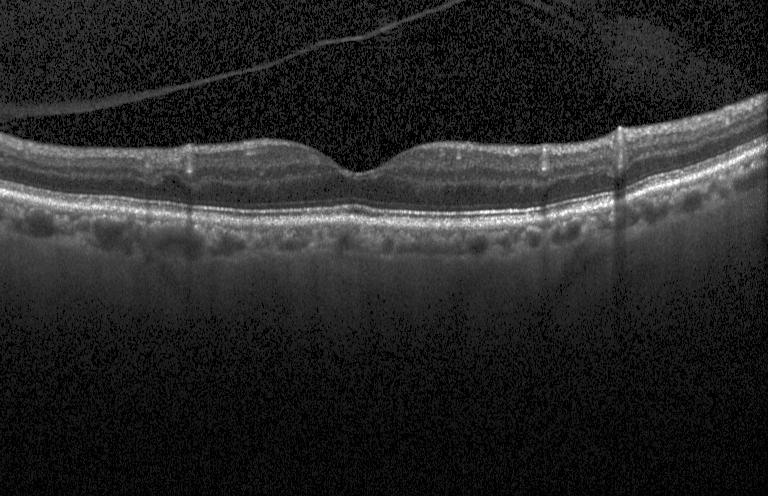
OCT B-scan.
No CNV, DME, or drusen.